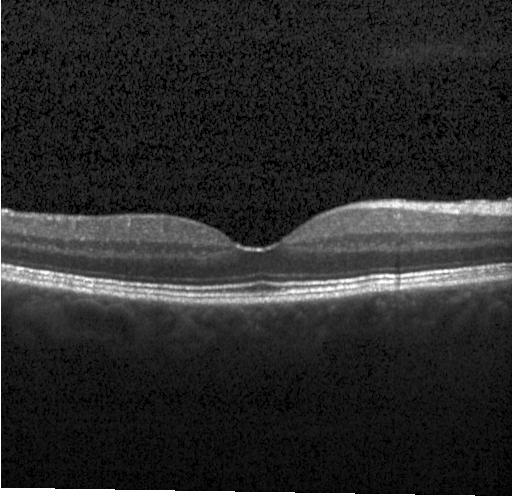
Horizontal scan through the fovea; spectral-domain OCT; Heidelberg Spectralis; optical coherence tomography B-scan. Assessment: neither choroidal neovascularization, diabetic macular edema, nor drusen.